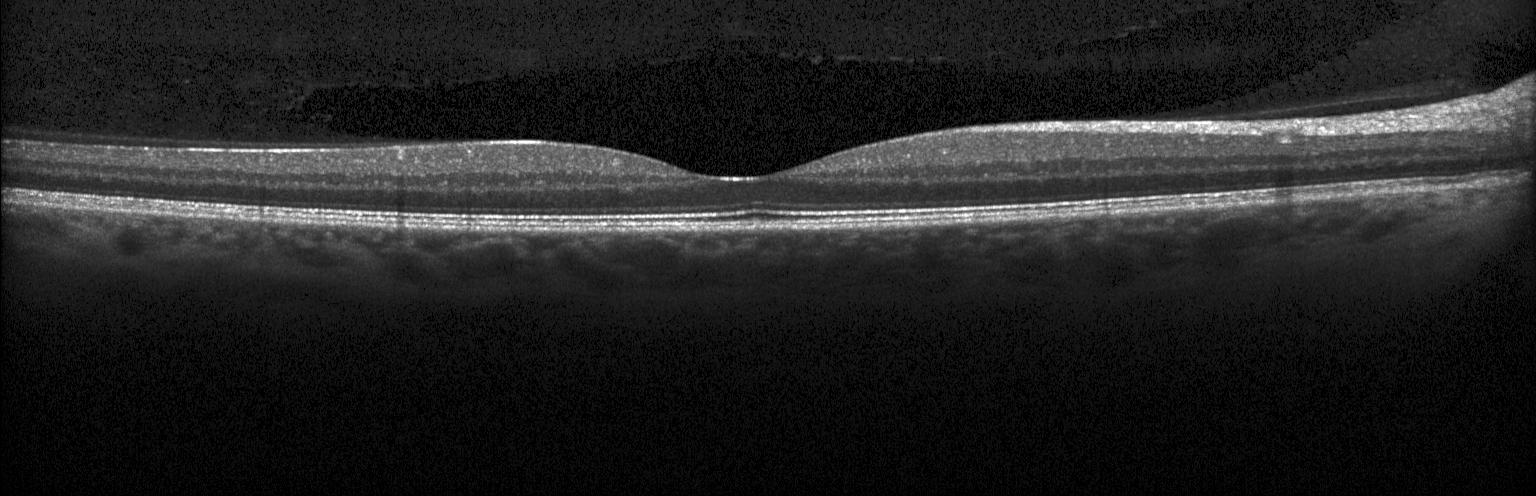

OCT scan showing no CNV, DME, or drusen.